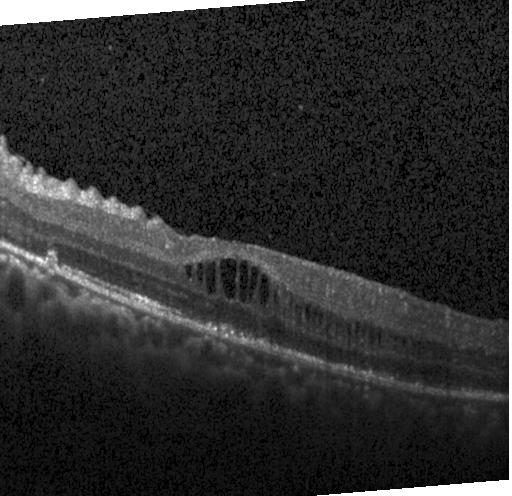

Diabetic macular edema.